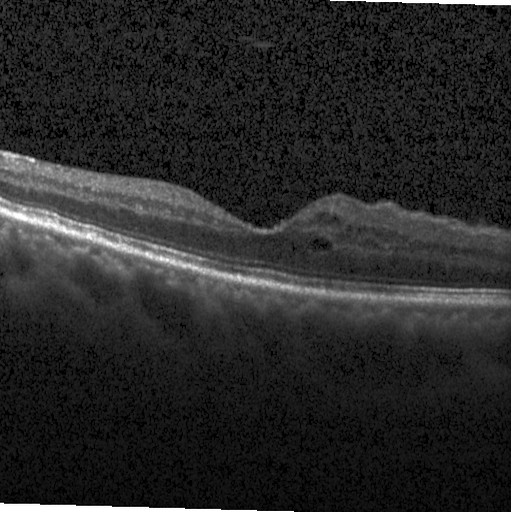

Acquired on a Heidelberg Spectralis. Optical coherence tomography scan. This B-scan demonstrates DME.